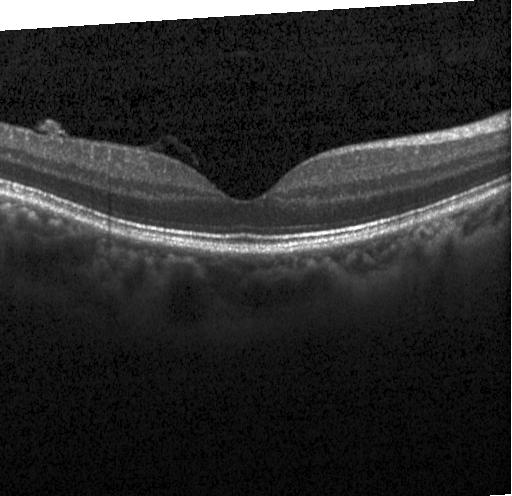 Finding: no choroidal neovascularization, no diabetic macular edema, and no drusen.